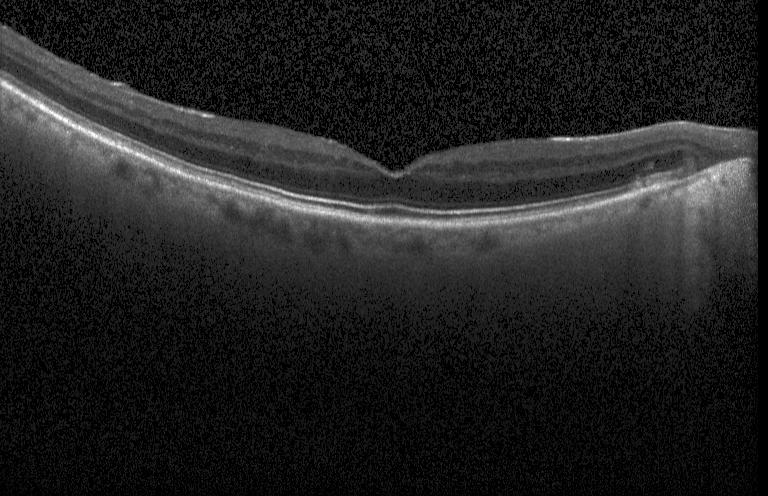 OCT B-scan, spectral-domain OCT, horizontal scan through the fovea, Heidelberg Spectralis OCT system.
Assessment: no choroidal neovascularization, no diabetic macular edema, and no drusen.